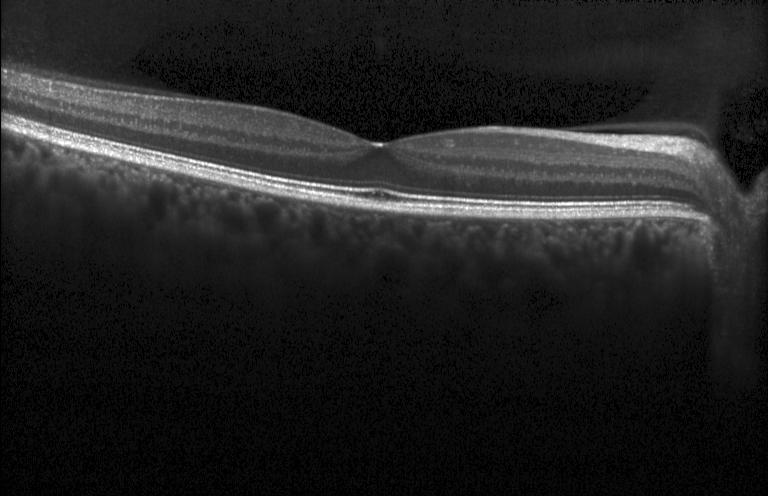

Retinal OCT cross-section; Heidelberg Spectralis; through the macula. Impression: no choroidal neovascularization, no diabetic macular edema, and no drusen.